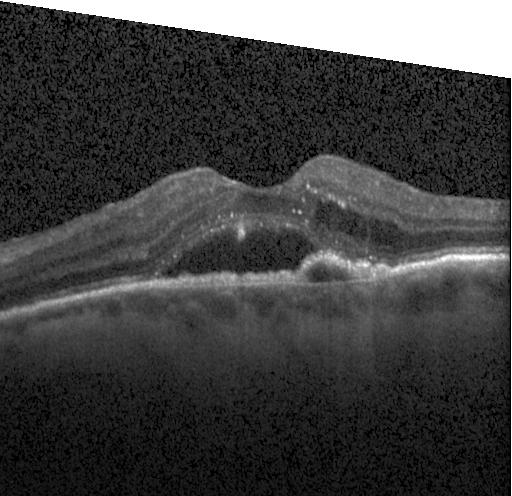
Optical coherence tomography B-scan.
The scan shows a choroidal neovascular membrane.